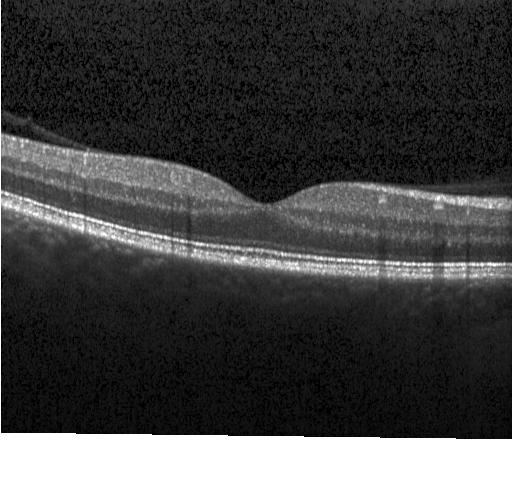 Optical coherence tomography scan — Impression: no choroidal neovascularization, no diabetic macular edema, and no drusen.